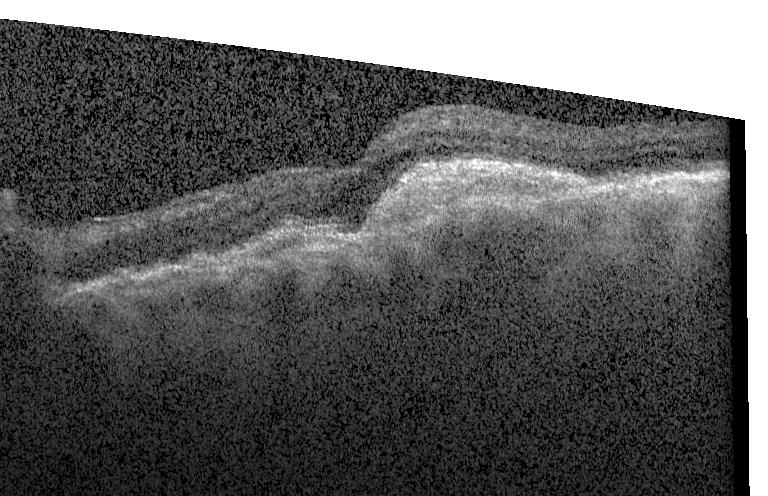 OCT B-scan. Heidelberg Spectralis. Fovea-centered — Impression: a choroidal neovascular membrane.